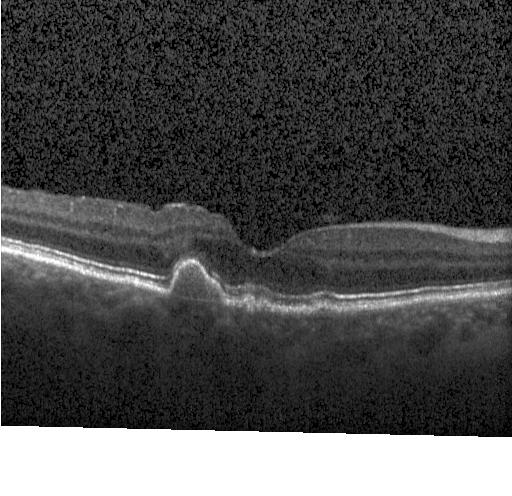
Horizontal scan through the fovea; OCT B-scan; acquired on a Heidelberg Spectralis
Impression: drusen.